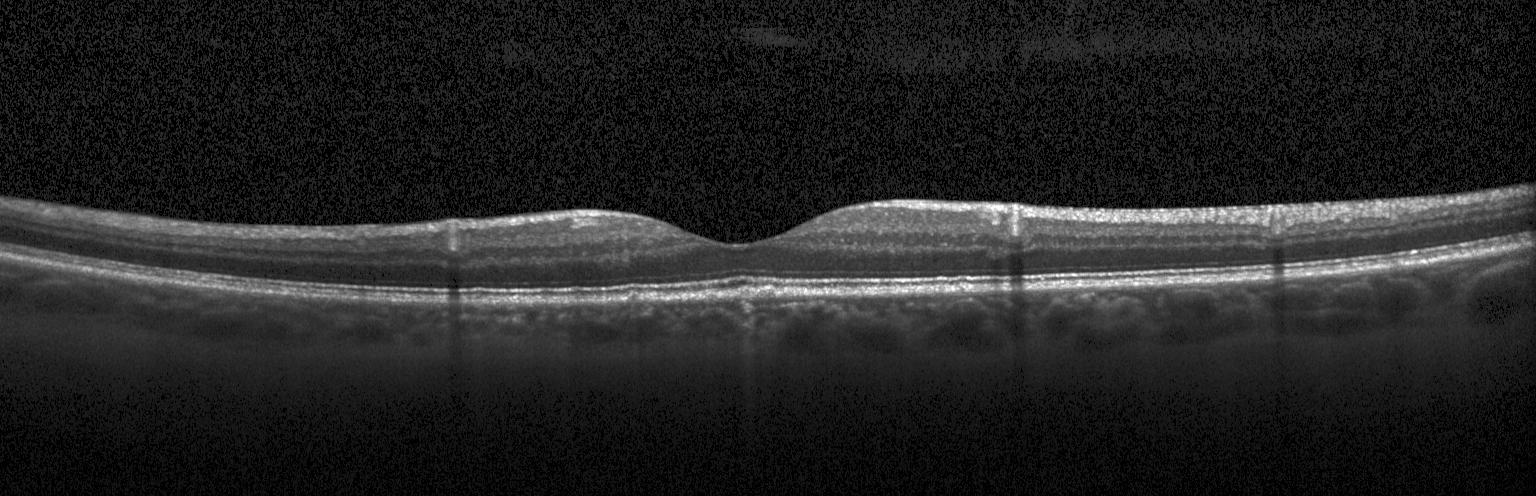

OCT B-scan; spectral-domain optical coherence tomography; macular scan; acquired on a Heidelberg Spectralis.
Dx: drusen.